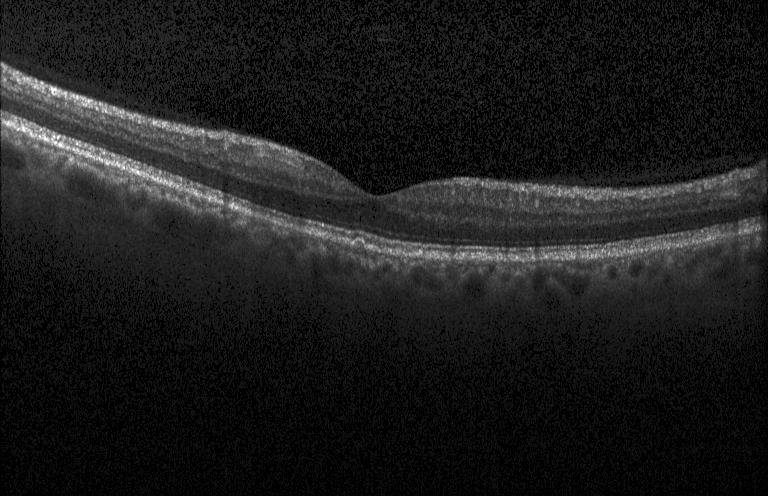 Finding: no choroidal neovascularization, no diabetic macular edema, and no drusen.